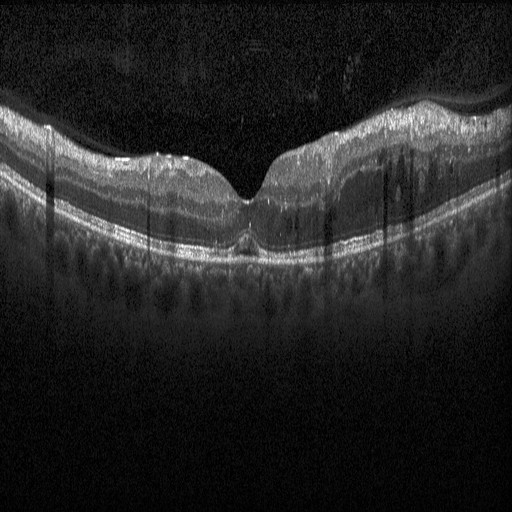
OCT line scan — Assessment: diabetic macular edema.